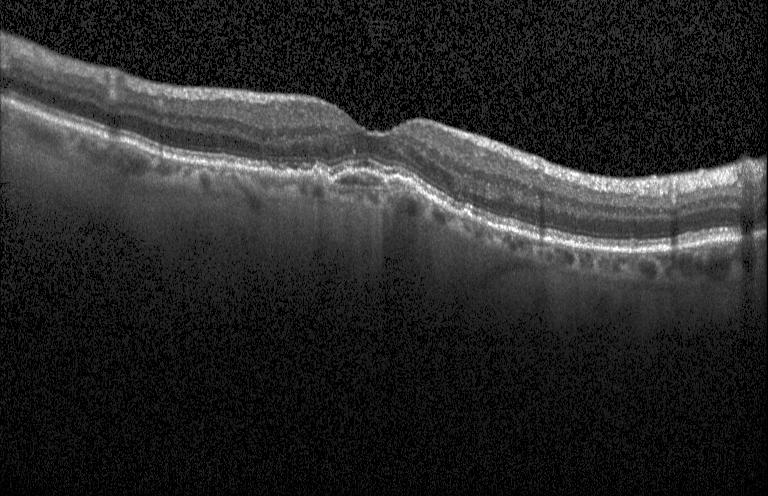

Through the macula; optical coherence tomography scan — Assessment: choroidal neovascularization.